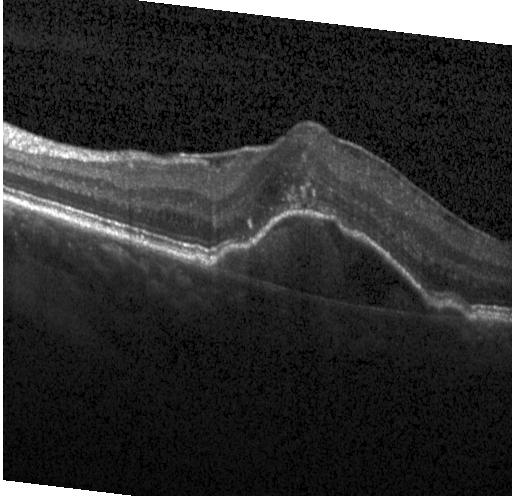

Impression: a choroidal neovascular membrane.